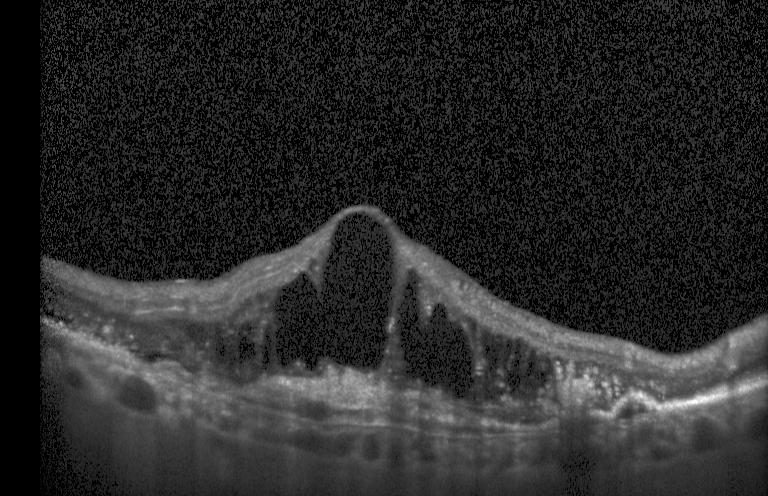
SD-OCT, OCT line scan, fovea-centered
This B-scan demonstrates a choroidal neovascular membrane.